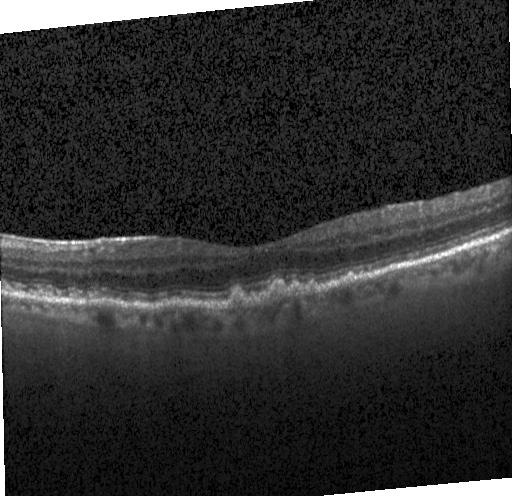

OCT finding: drusen.